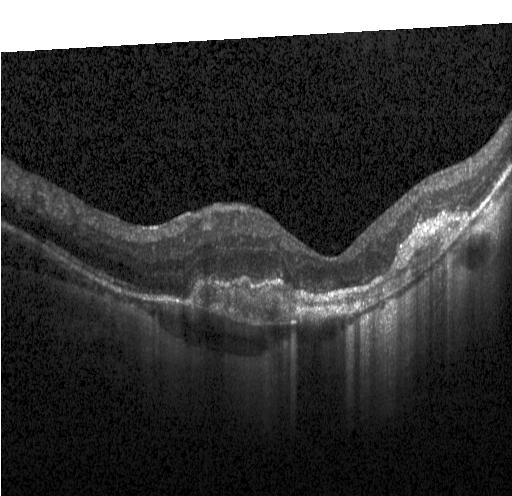 Retinal OCT B-scan. Macular scan. Spectral-domain optical coherence tomography. Heidelberg Spectralis OCT system.
Assessment: a choroidal neovascular membrane.